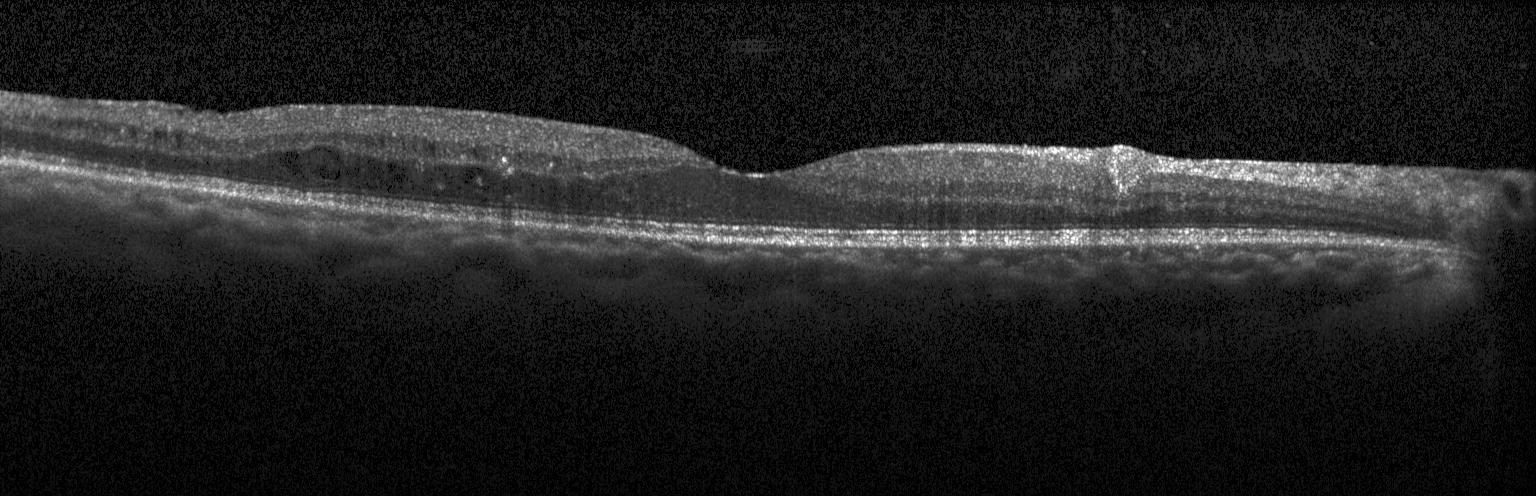

OCT finding: diabetic macular edema.